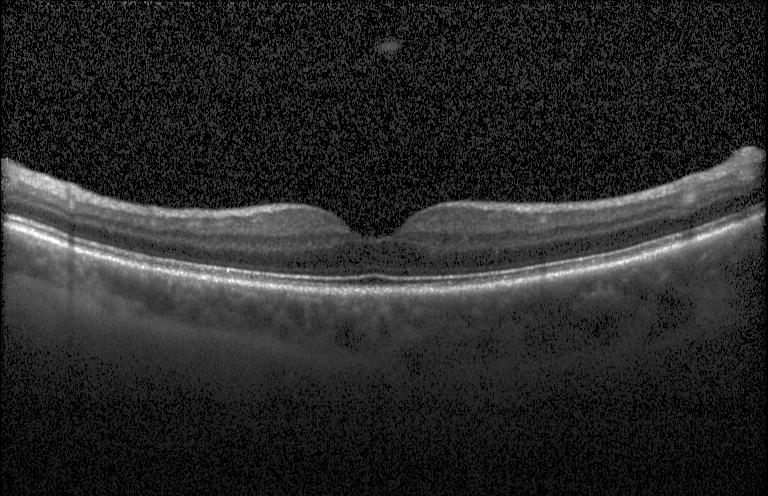

No evidence of choroidal neovascularization, diabetic macular edema, or drusen.